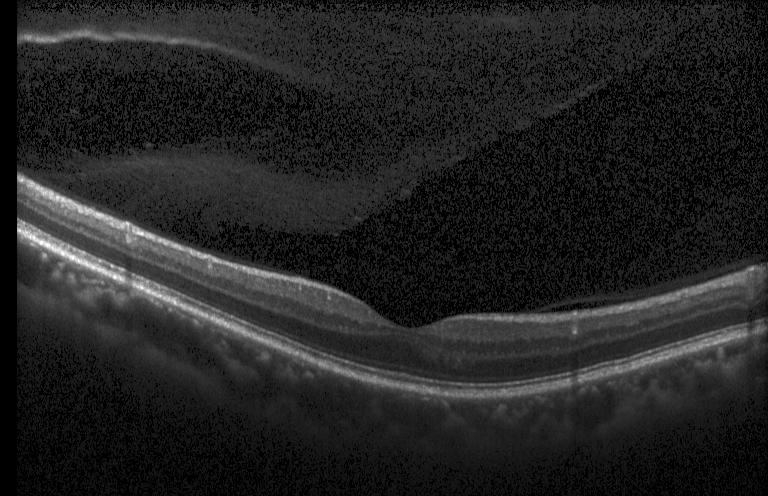
Retinal OCT B-scan · SD-OCT · horizontal scan through the fovea
Impression: neither CNV, DME, nor drusen.